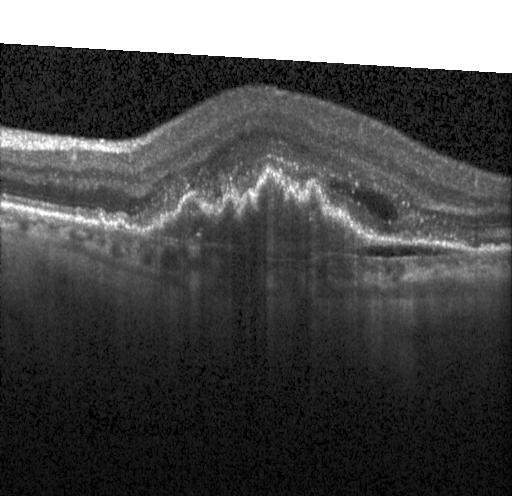 SD-OCT, retinal OCT cross-section.
Finding: choroidal neovascularization (CNV).